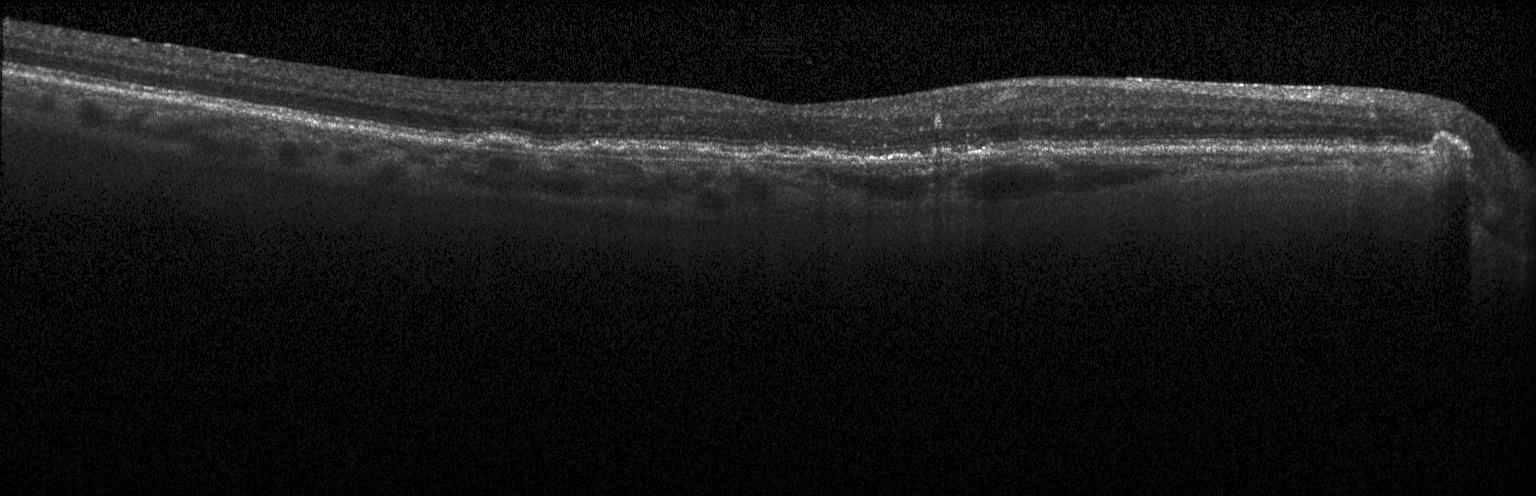

SD-OCT; through the macula; OCT line scan — This B-scan demonstrates choroidal neovascularization.